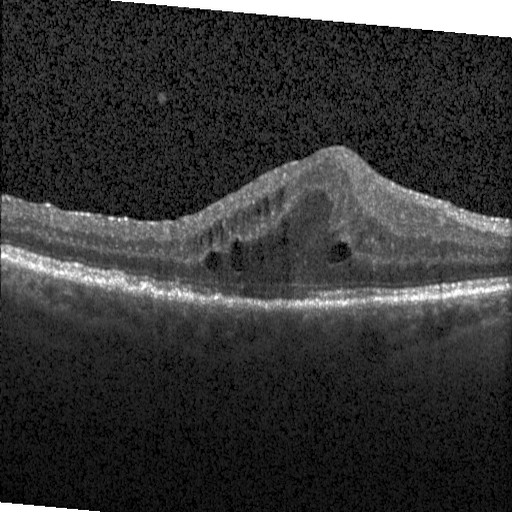

This B-scan demonstrates diabetic macular edema (DME).